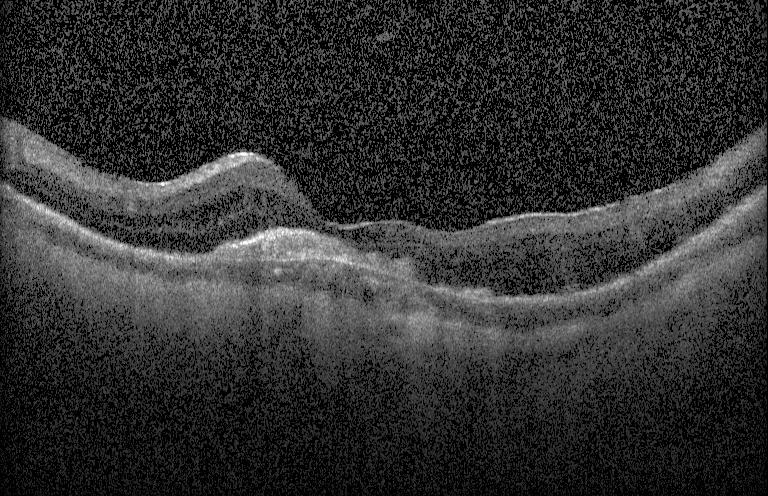

Fovea-centered · OCT line scan
The scan shows choroidal neovascularization.